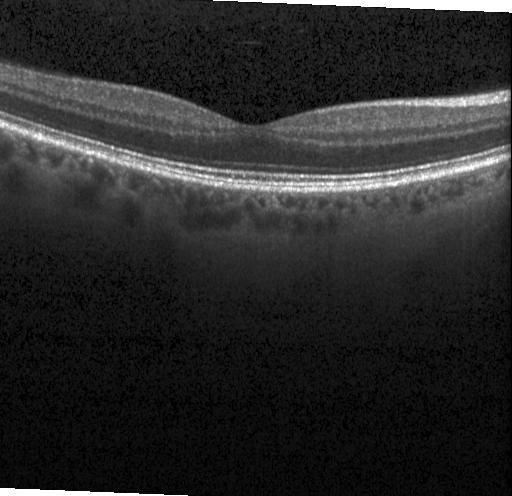

Diagnosis: no choroidal neovascularization, no diabetic macular edema, and no drusen.